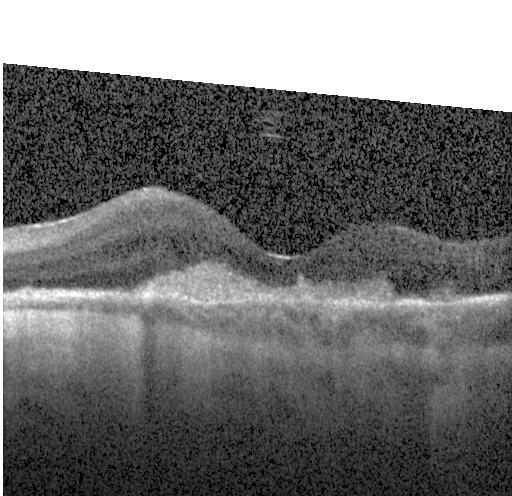 Impression: a choroidal neovascular membrane.